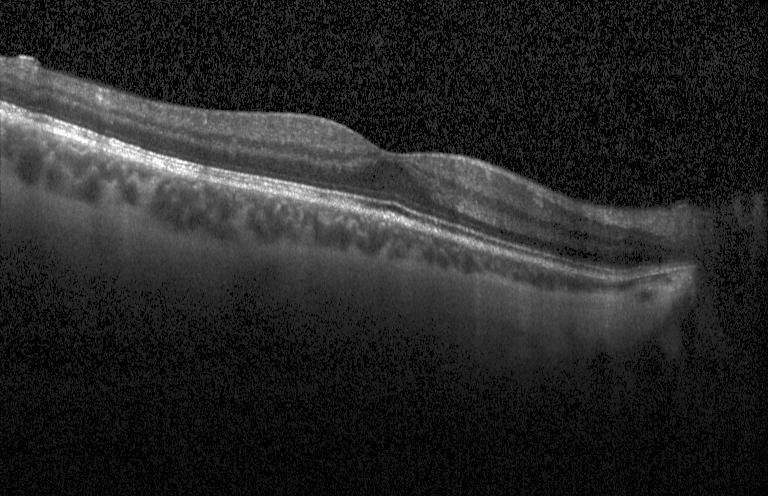 Through the macula · optical coherence tomography B-scan · Heidelberg Spectralis · spectral-domain OCT. Dx: neither CNV, DME, nor drusen.